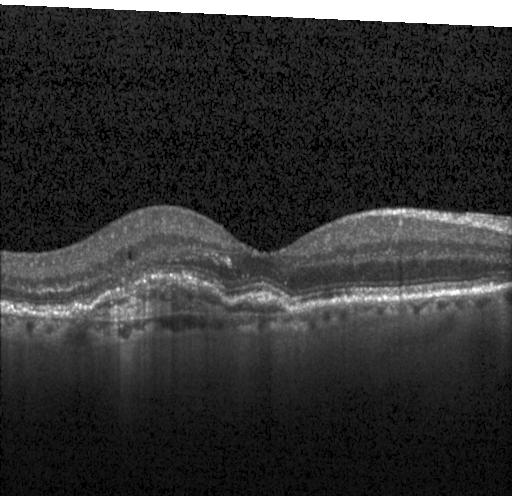
Optical coherence tomography B-scan
Impression: a choroidal neovascular membrane.